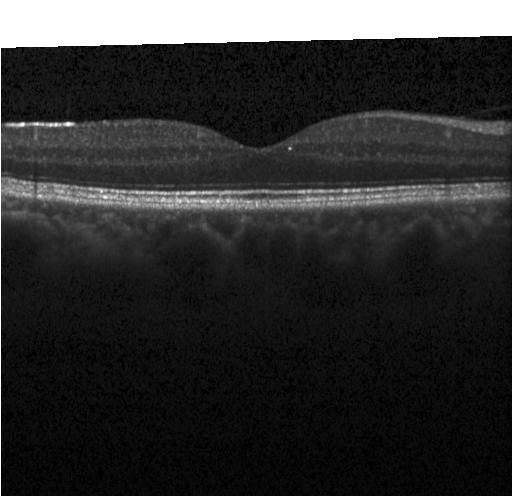

Impression: neither choroidal neovascularization, diabetic macular edema, nor drusen.